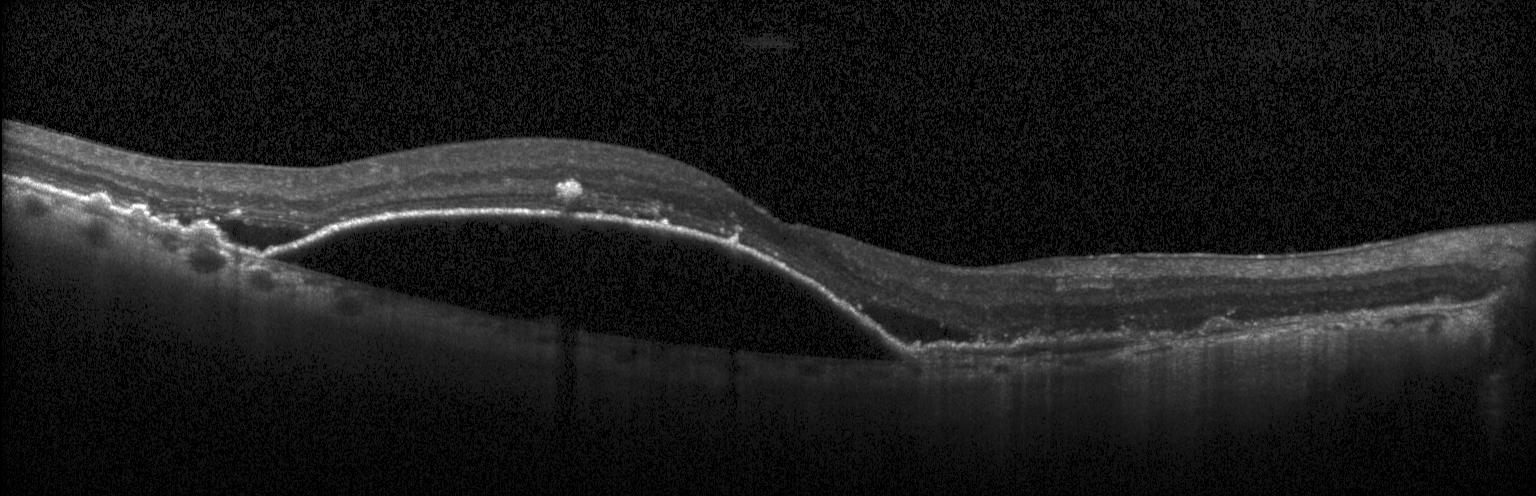
Macular scan · retinal OCT B-scan
The scan shows choroidal neovascularization (CNV).